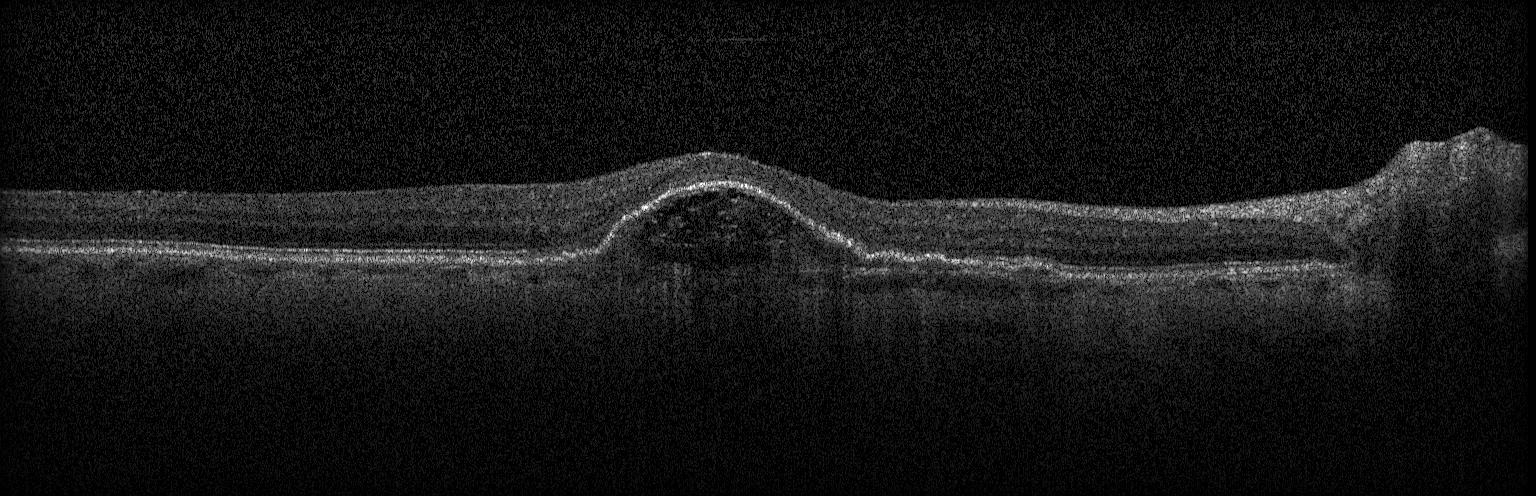 Retinal OCT cross-section showing a choroidal neovascular membrane.